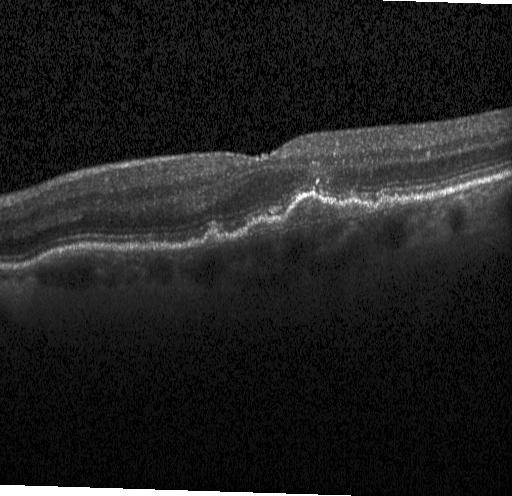 Retinal OCT B-scan; through the macula
This B-scan demonstrates choroidal neovascularization (CNV).